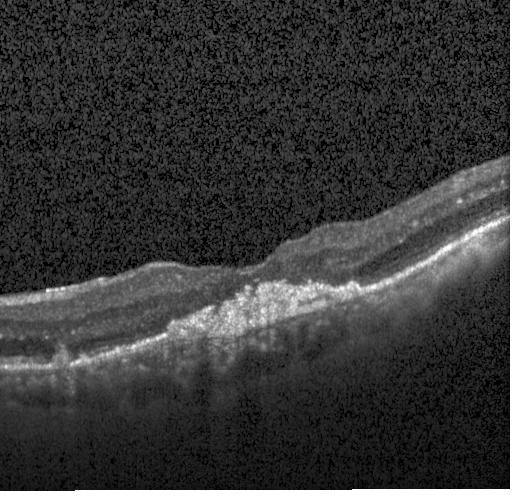

Diagnosis: a choroidal neovascular membrane.